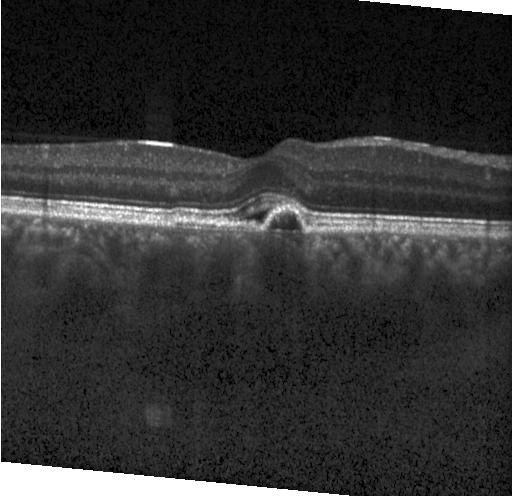
OCT B-scan. Heidelberg Spectralis OCT system. Spectral-domain OCT. Horizontal scan through the fovea — Diagnosis: choroidal neovascularization (CNV).